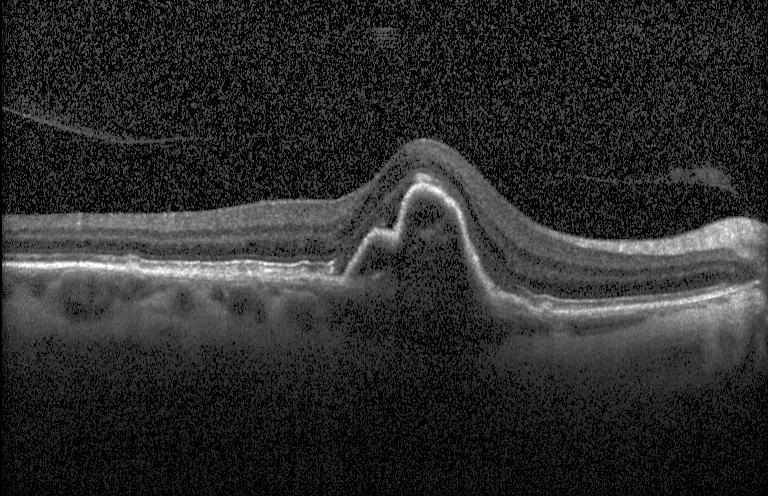 OCT B-scan.
Assessment: choroidal neovascularization (CNV).